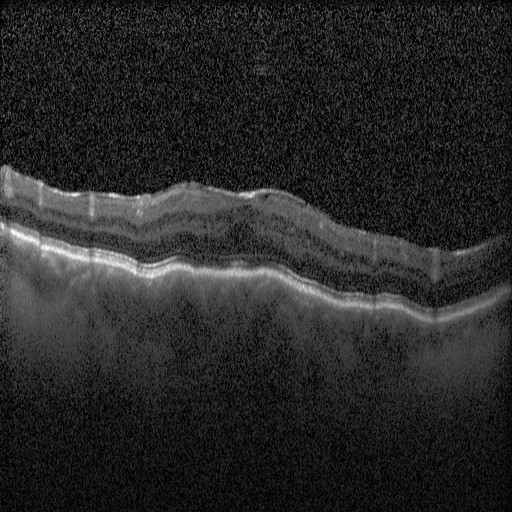
Macular scan. Optical coherence tomography scan. Spectral-domain OCT. Instrument: Heidelberg Spectralis
Impression: diabetic macular edema.